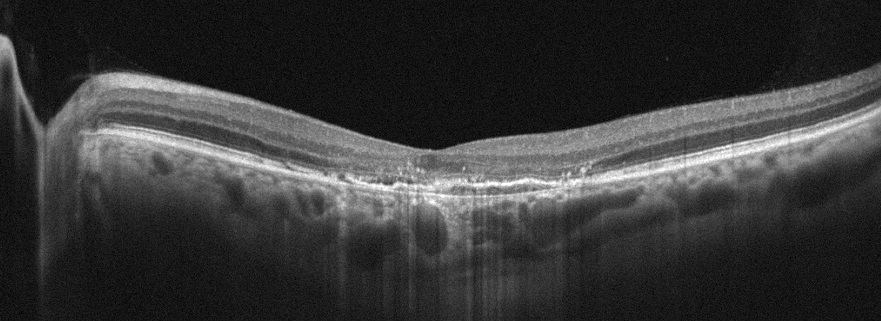

Diagnosis: age-related macular degeneration.